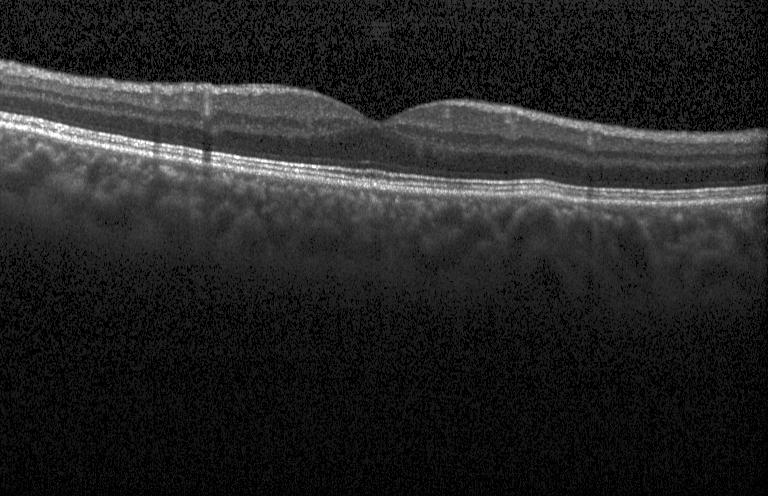 Impression: no evidence of choroidal neovascularization, diabetic macular edema, or drusen.